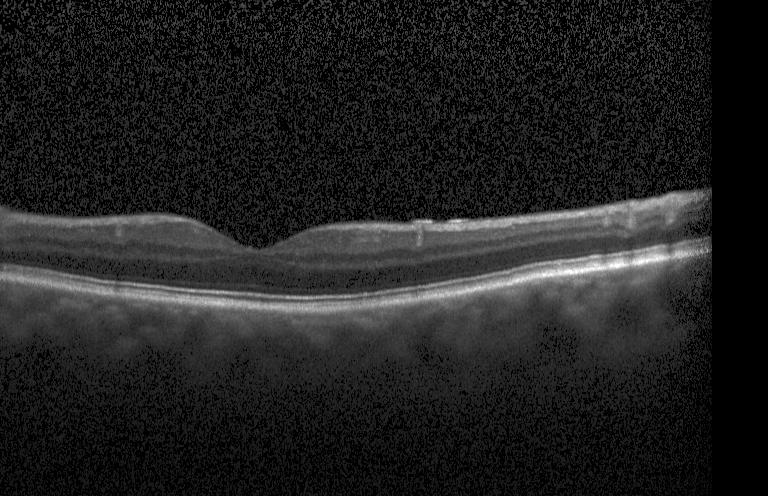 Heidelberg Spectralis OCT system. Retinal OCT cross-section
Assessment: neither choroidal neovascularization, diabetic macular edema, nor drusen.